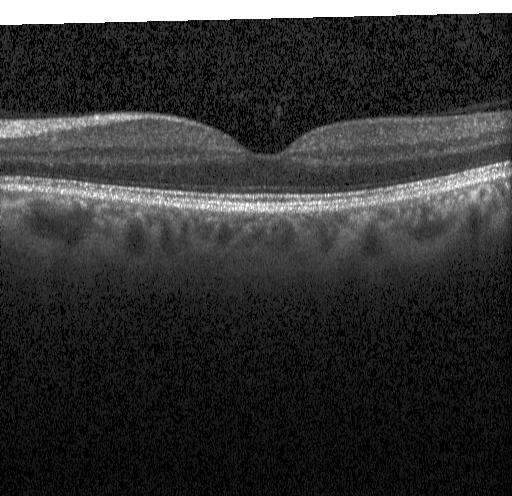 Retinal OCT B-scan. Assessment: neither CNV, DME, nor drusen.